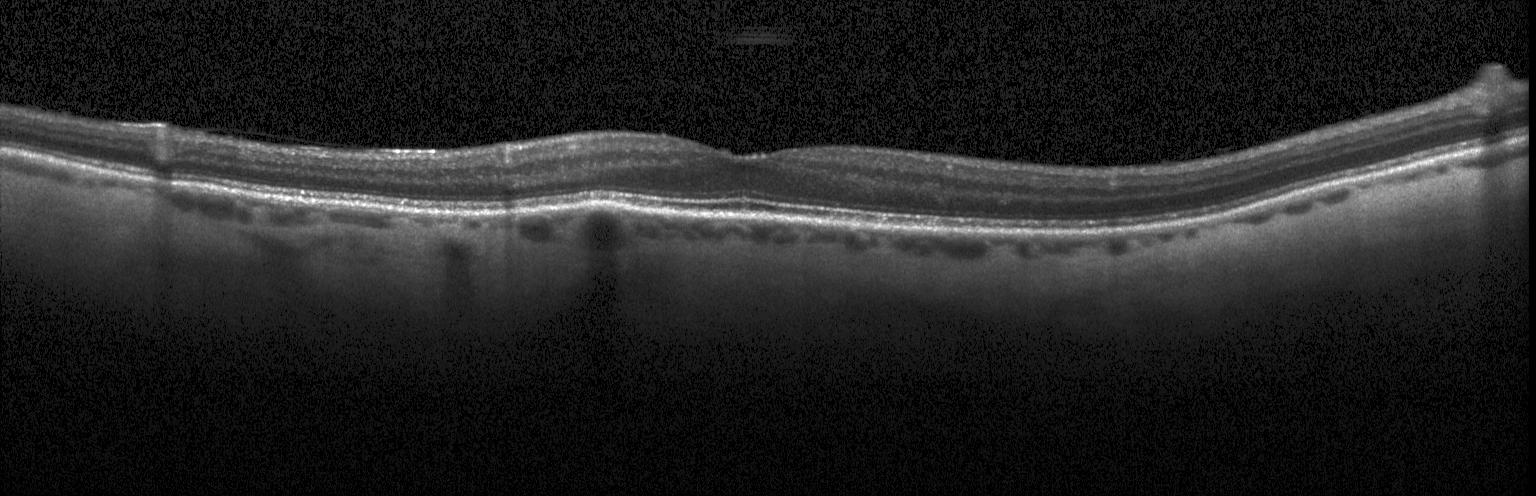
Macular scan · Heidelberg Spectralis OCT system · retinal OCT B-scan
OCT finding: no choroidal neovascularization, no diabetic macular edema, and no drusen.